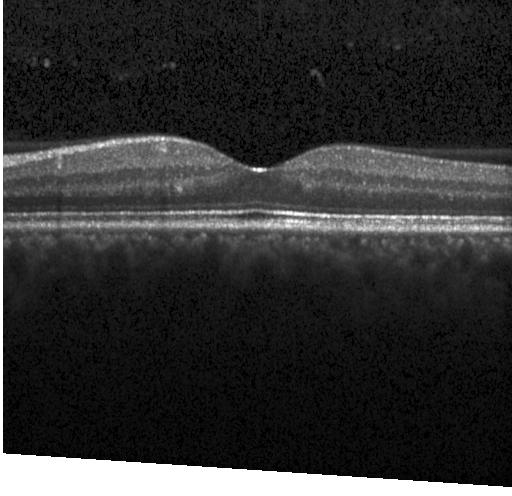

No choroidal neovascularization, no diabetic macular edema, and no drusen.